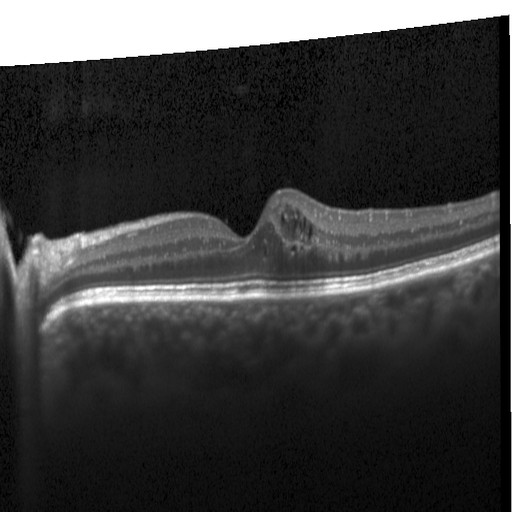

Heidelberg Spectralis OCT system · SD-OCT · fovea-centered · retinal OCT cross-section.
Dx: diabetic macular edema (DME).